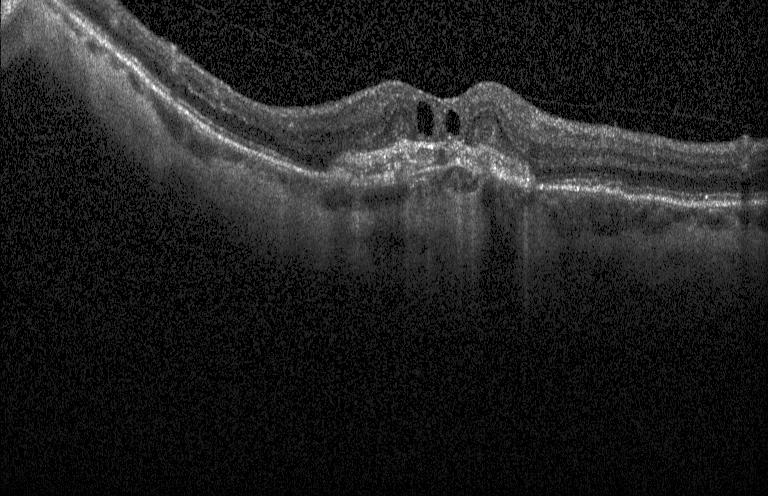 Retinal OCT cross-section showing a choroidal neovascular membrane.